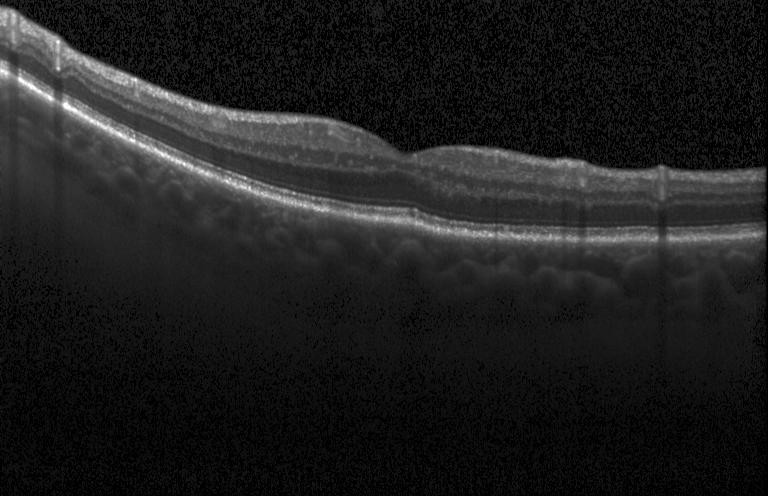 Diagnosis: no choroidal neovascularization, no diabetic macular edema, and no drusen.